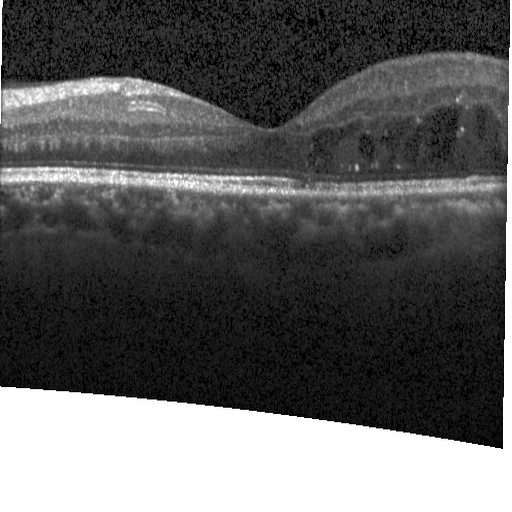
Macular OCT demonstrating diabetic macular edema.